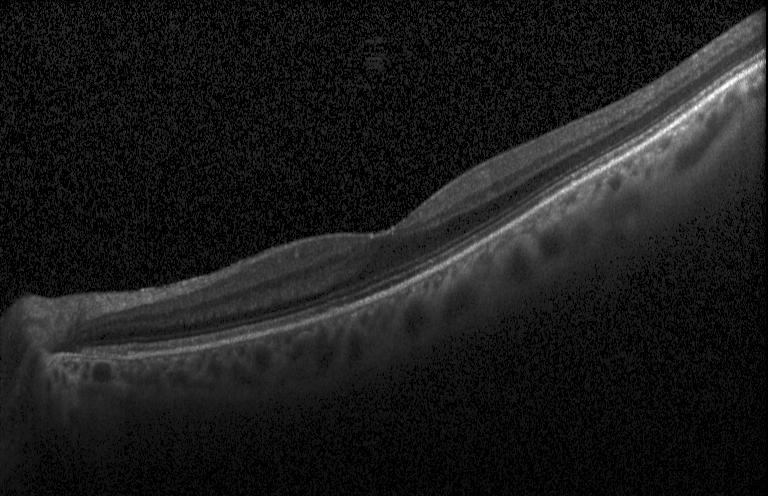
No evidence of choroidal neovascularization, diabetic macular edema, or drusen.